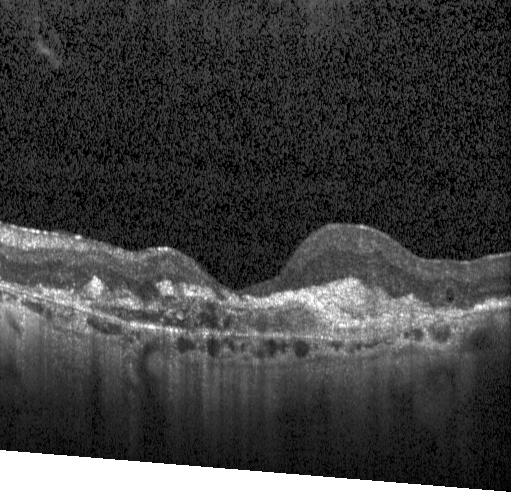
Diagnosis: choroidal neovascularization (CNV).